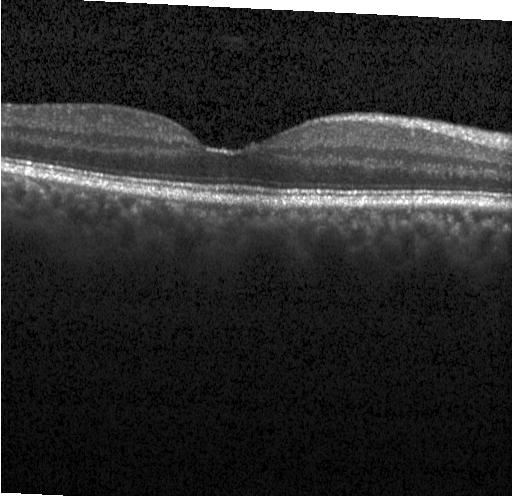
Spectral-domain optical coherence tomography, retinal OCT B-scan, instrument: Heidelberg Spectralis.
Diagnosis: no choroidal neovascularization, no diabetic macular edema, and no drusen.